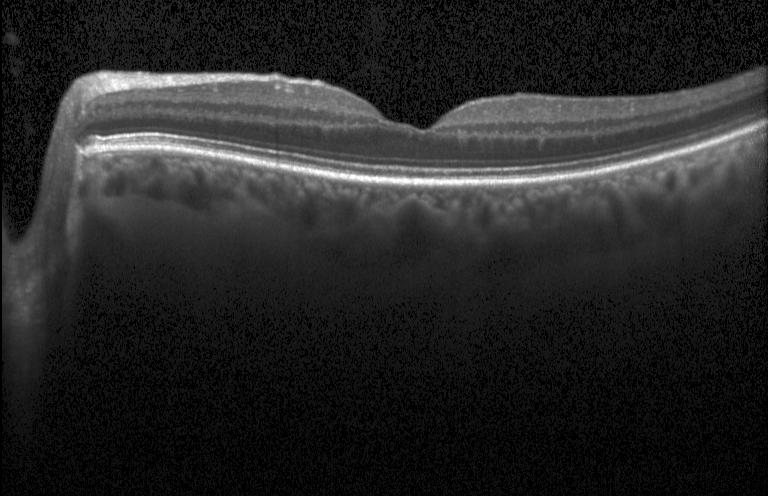
OCT B-scan
This B-scan demonstrates no choroidal neovascularization, diabetic macular edema, or drusen.